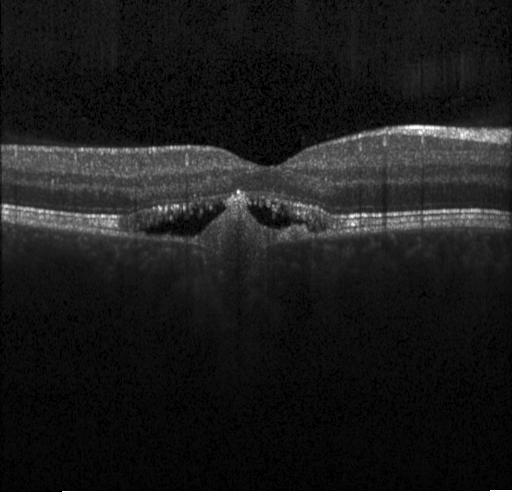 Heidelberg Spectralis · retinal OCT B-scan · SD-OCT.
Diagnosis: choroidal neovascularization.